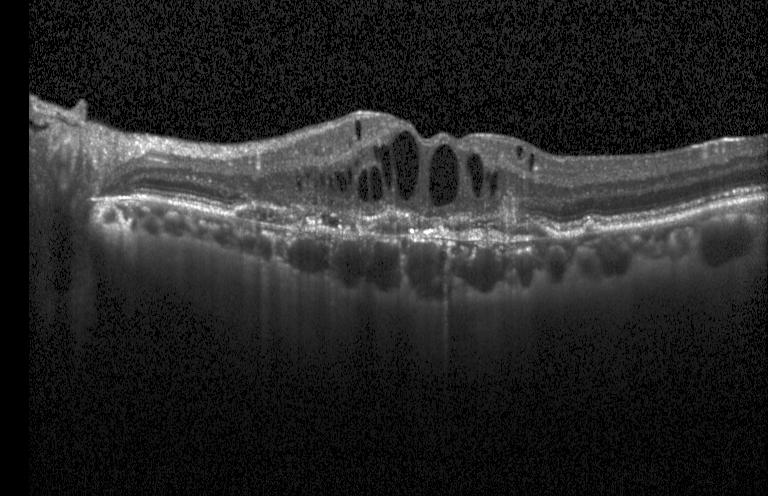

Finding: a choroidal neovascular membrane.